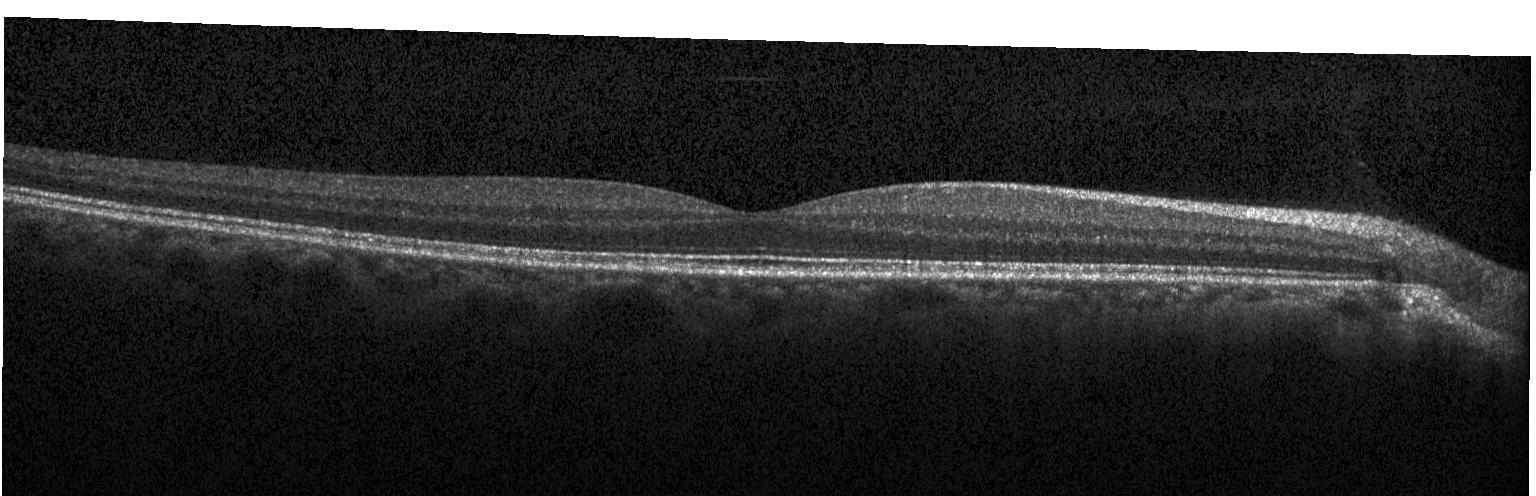

Spectral-domain OCT; OCT line scan; instrument: Heidelberg Spectralis; horizontal scan through the fovea
Finding: neither choroidal neovascularization, diabetic macular edema, nor drusen.